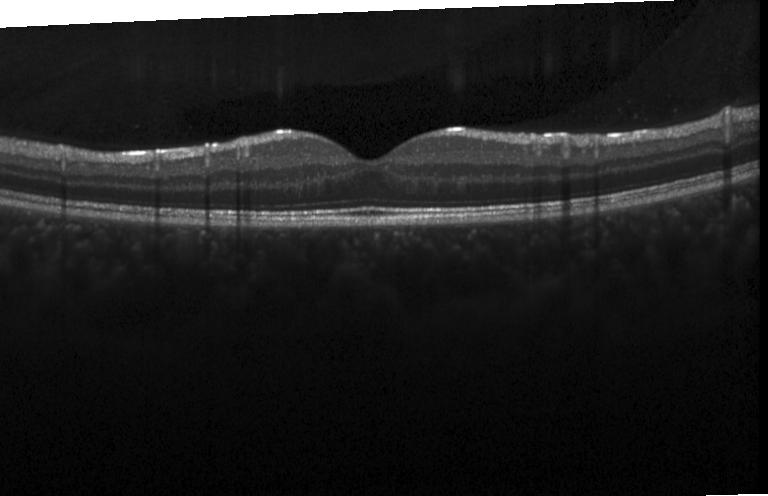
Spectral-domain OCT · optical coherence tomography B-scan — Diagnosis: no evidence of CNV, DME, or drusen.